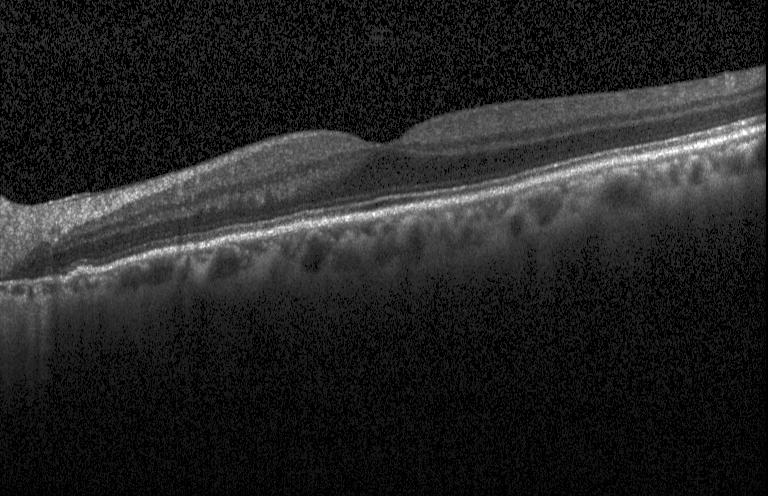
Spectral-domain OCT B-scan: no evidence of choroidal neovascularization, diabetic macular edema, or drusen.